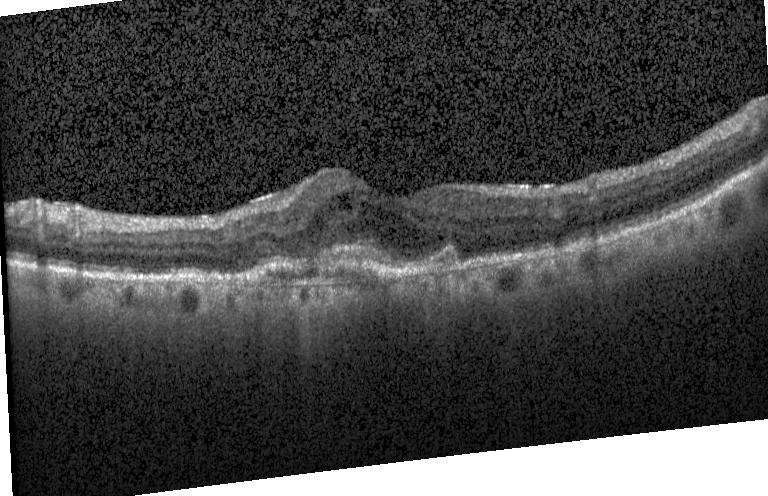
Finding: a choroidal neovascular membrane.